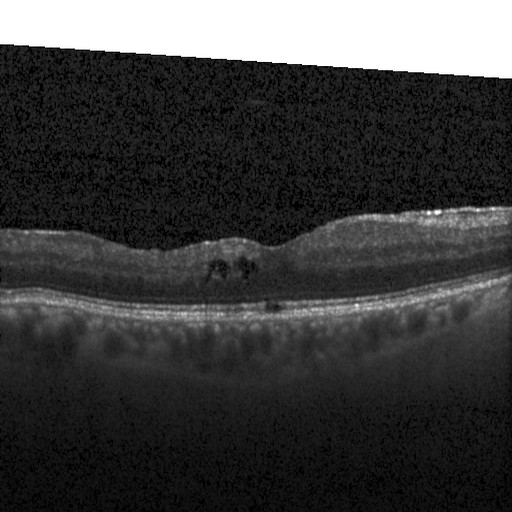 Through the macula · acquired on a Heidelberg Spectralis · SD-OCT · optical coherence tomography B-scan — Impression: diabetic macular edema (DME).